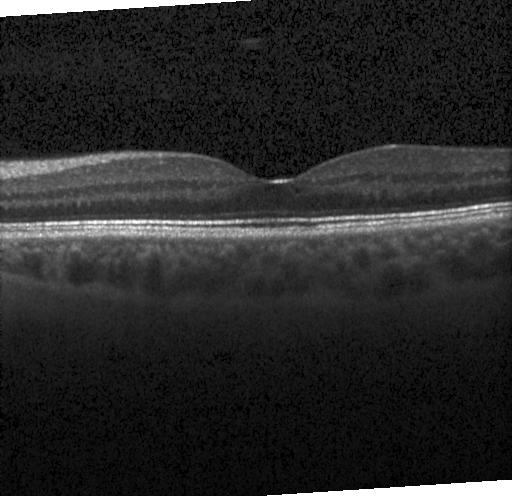 Centered on the fovea; retinal OCT B-scan. No CNV, no DME, and no drusen.